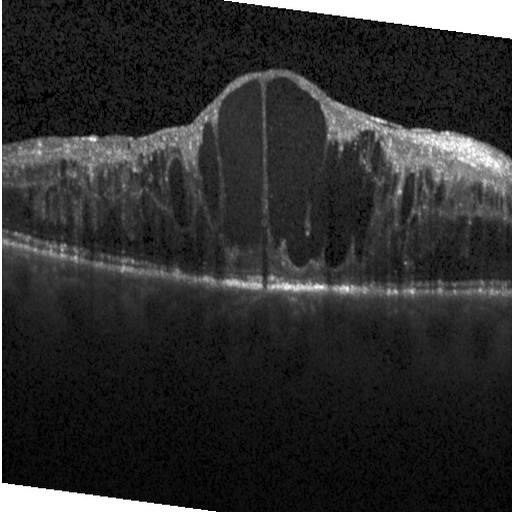 Spectral-domain OCT. Optical coherence tomography scan. Instrument: Heidelberg Spectralis. Horizontal scan through the fovea — Dx: DME.